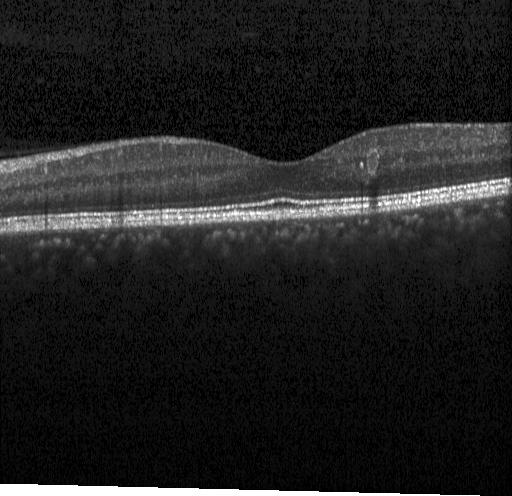

Heidelberg Spectralis; optical coherence tomography scan.
Macular OCT: neither choroidal neovascularization, diabetic macular edema, nor drusen.